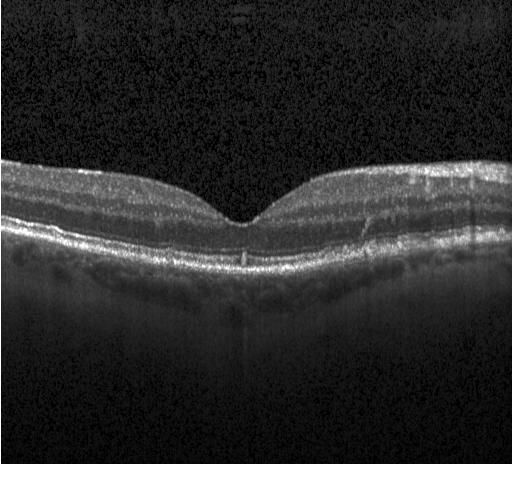 Diagnosis: sub-RPE drusenoid deposits.